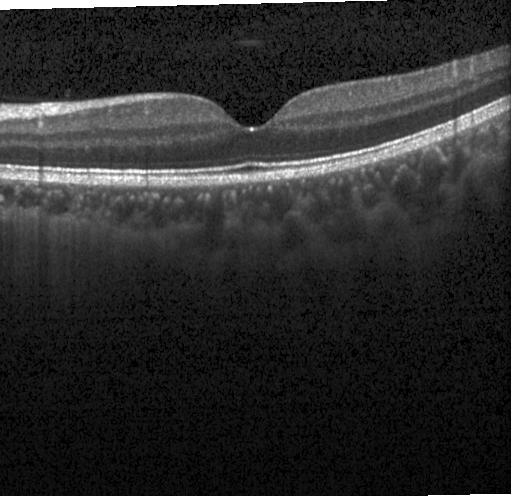
Macular OCT demonstrating no CNV, DME, or drusen.